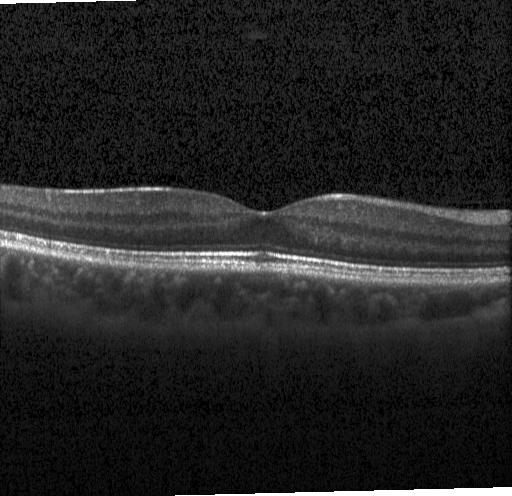
OCT line scan — Finding: neither choroidal neovascularization, diabetic macular edema, nor drusen.